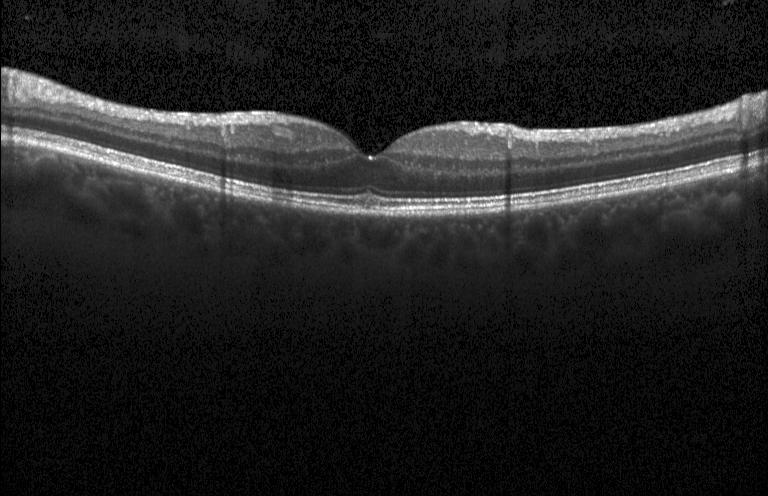 OCT finding: neither CNV, DME, nor drusen.